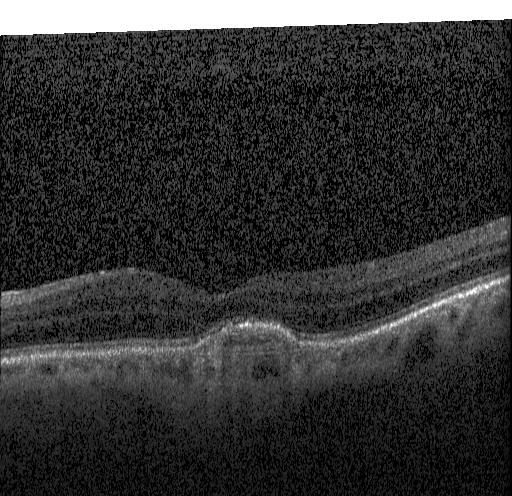
OCT line scan. Dx: choroidal neovascularization (CNV).